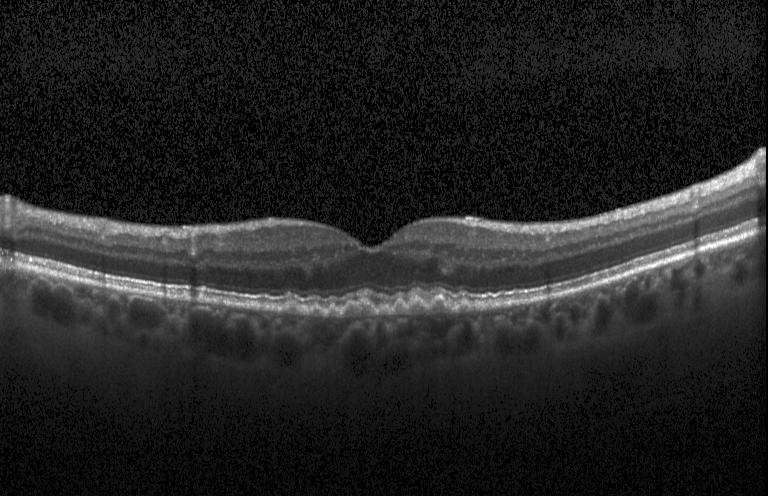 OCT line scan
Sub-RPE drusenoid deposits.